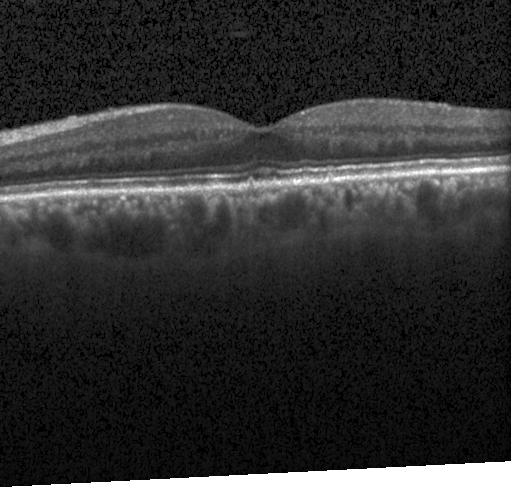 Heidelberg Spectralis OCT system; macular scan; retinal OCT cross-section; SD-OCT.
Drusen.